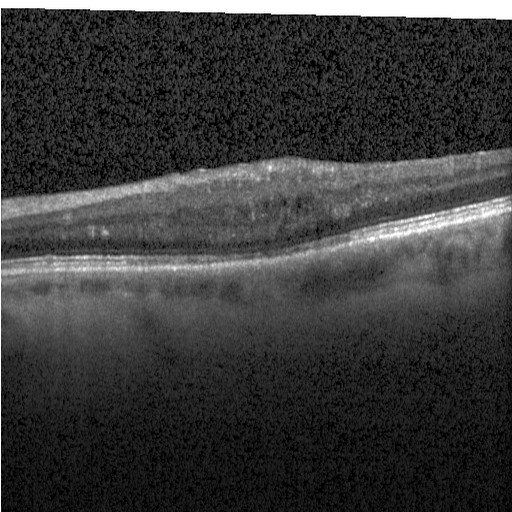

Retinal OCT B-scan. Assessment: DME.